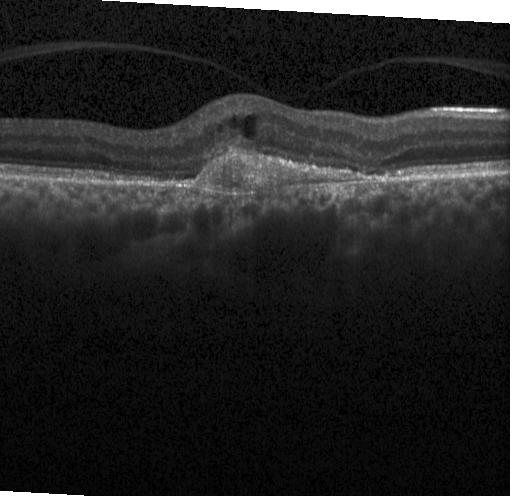
Diagnosis: a choroidal neovascular membrane.